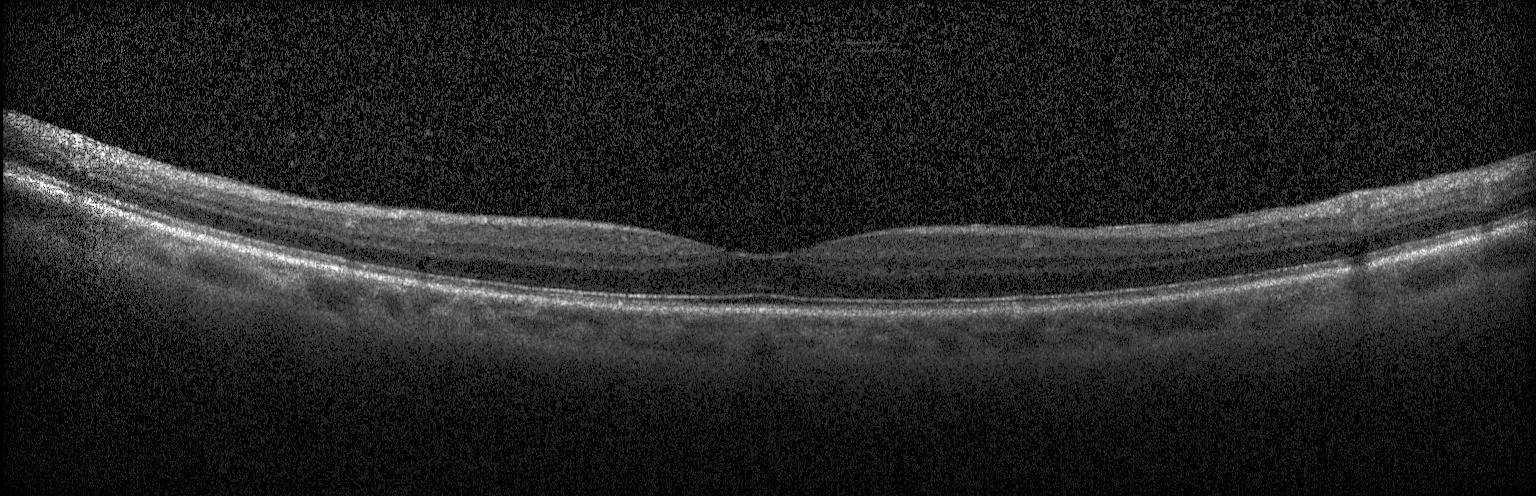 Spectral-domain optical coherence tomography · OCT B-scan · Heidelberg Spectralis OCT system · horizontal scan through the fovea
Assessment: no evidence of CNV, DME, or drusen.